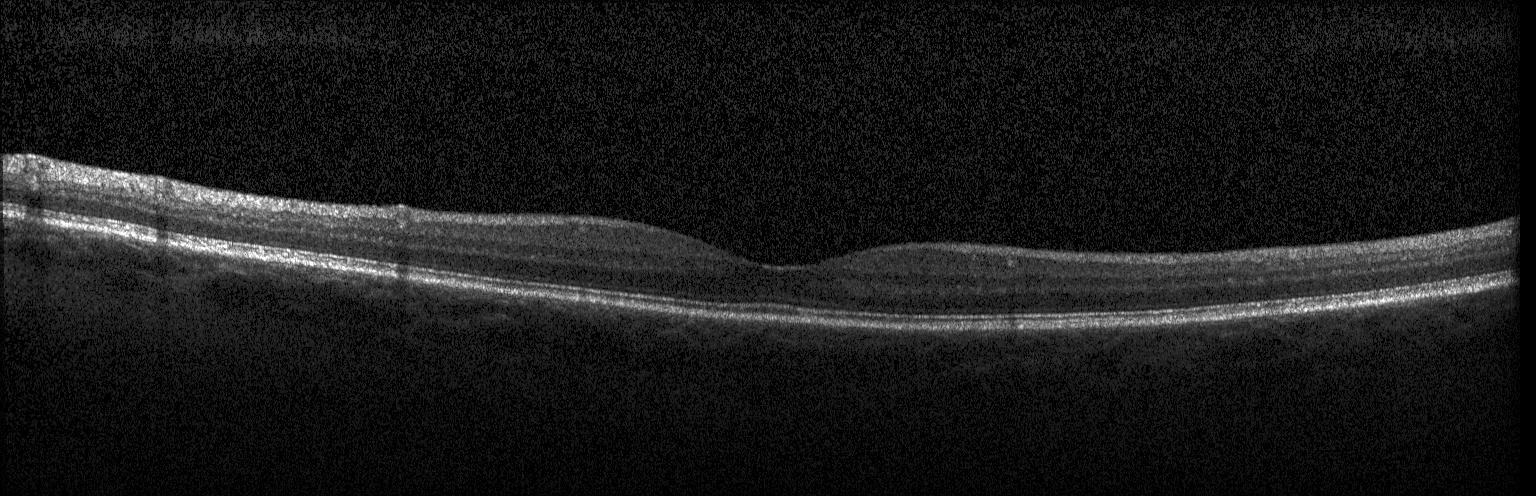 This B-scan demonstrates no evidence of choroidal neovascularization, diabetic macular edema, or drusen.